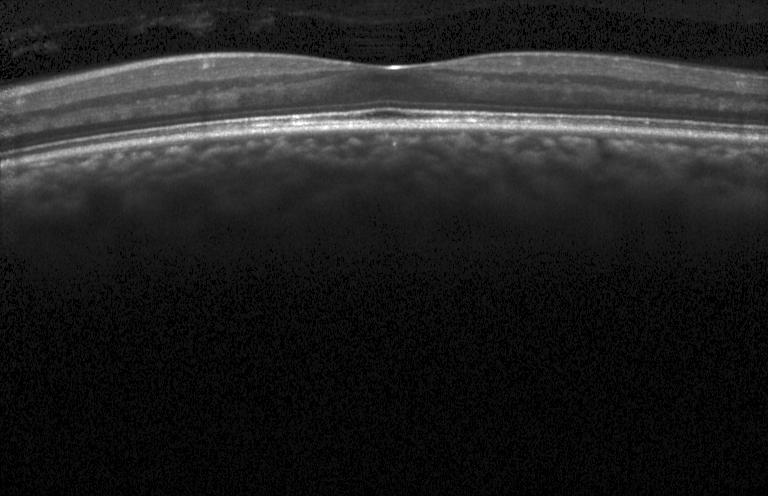

OCT B-scan showing no CNV, no DME, and no drusen.